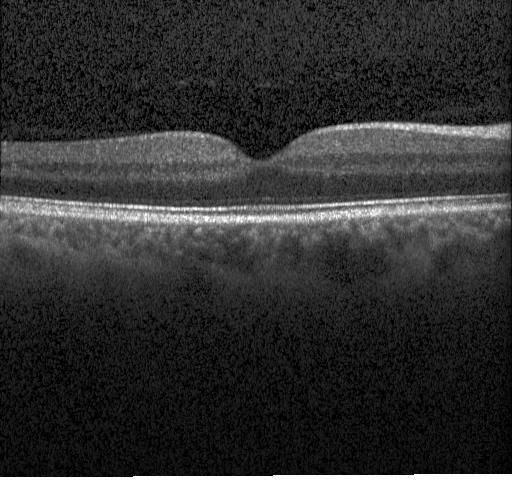

Macular OCT demonstrating no choroidal neovascularization, no diabetic macular edema, and no drusen.